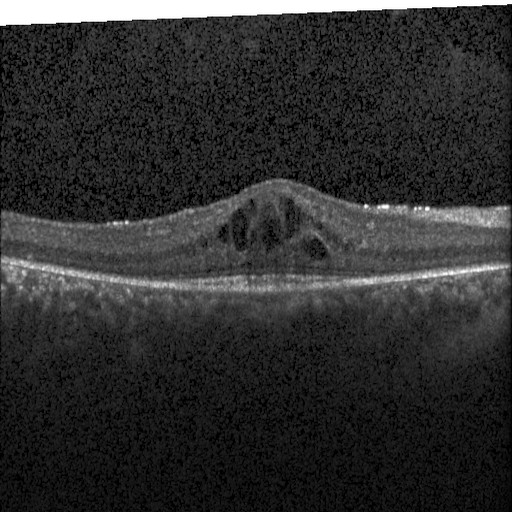 Acquired on a Heidelberg Spectralis; retinal OCT B-scan; SD-OCT. Macular OCT: diabetic macular edema.